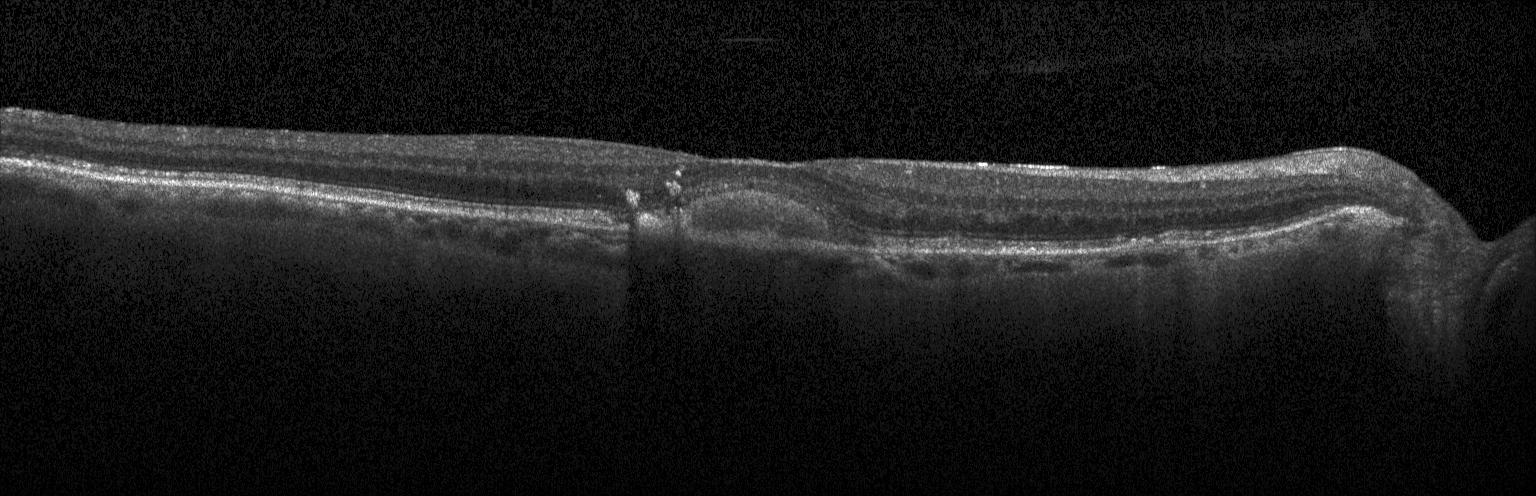
OCT B-scan · horizontal scan through the fovea · spectral-domain OCT. Impression: CNV.